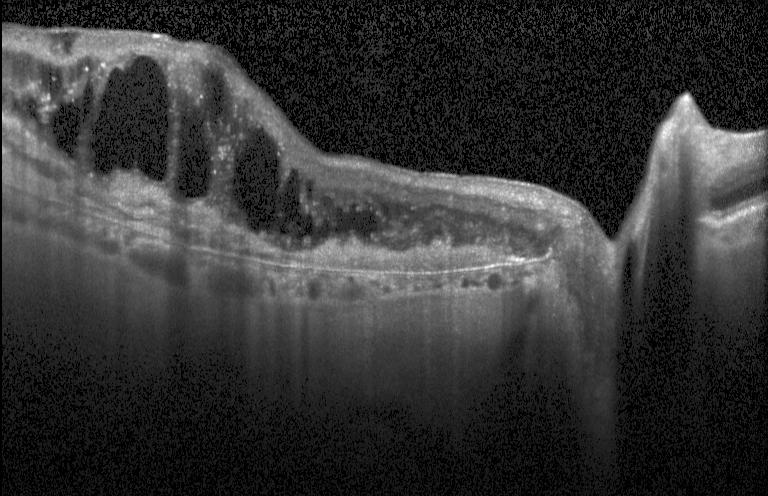
OCT line scan
This B-scan demonstrates a choroidal neovascular membrane.